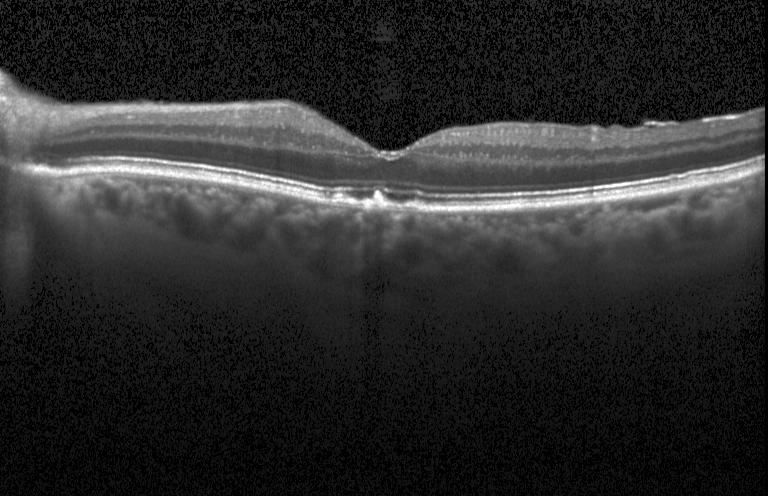

OCT B-scan showing multiple drusen.